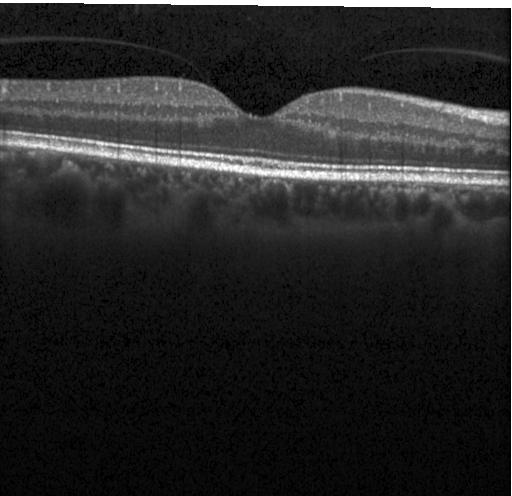
Centered on the fovea. Retinal OCT cross-section — This B-scan demonstrates no choroidal neovascularization, diabetic macular edema, or drusen.